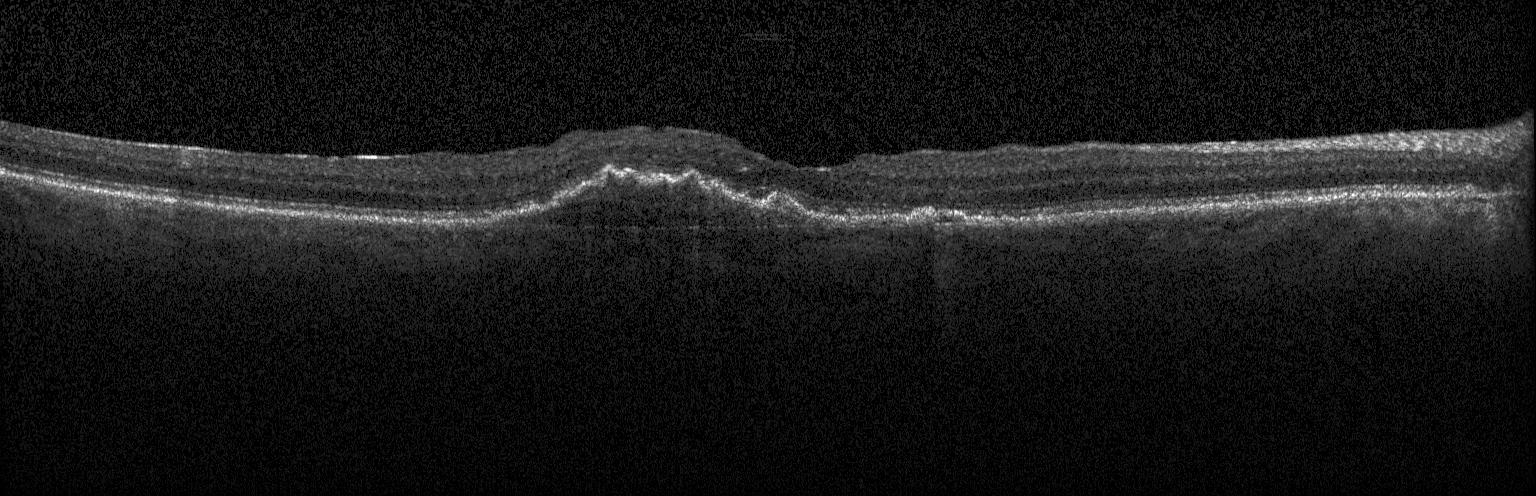 A choroidal neovascular membrane.